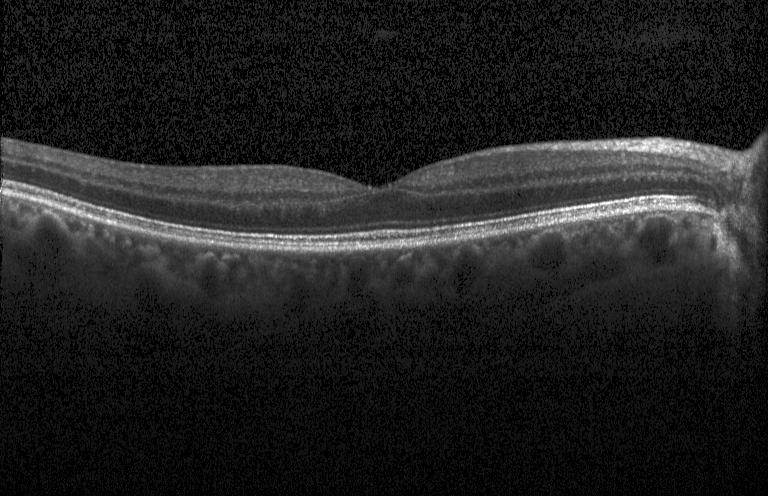
Retinal OCT cross-section — Dx: no evidence of choroidal neovascularization, diabetic macular edema, or drusen.